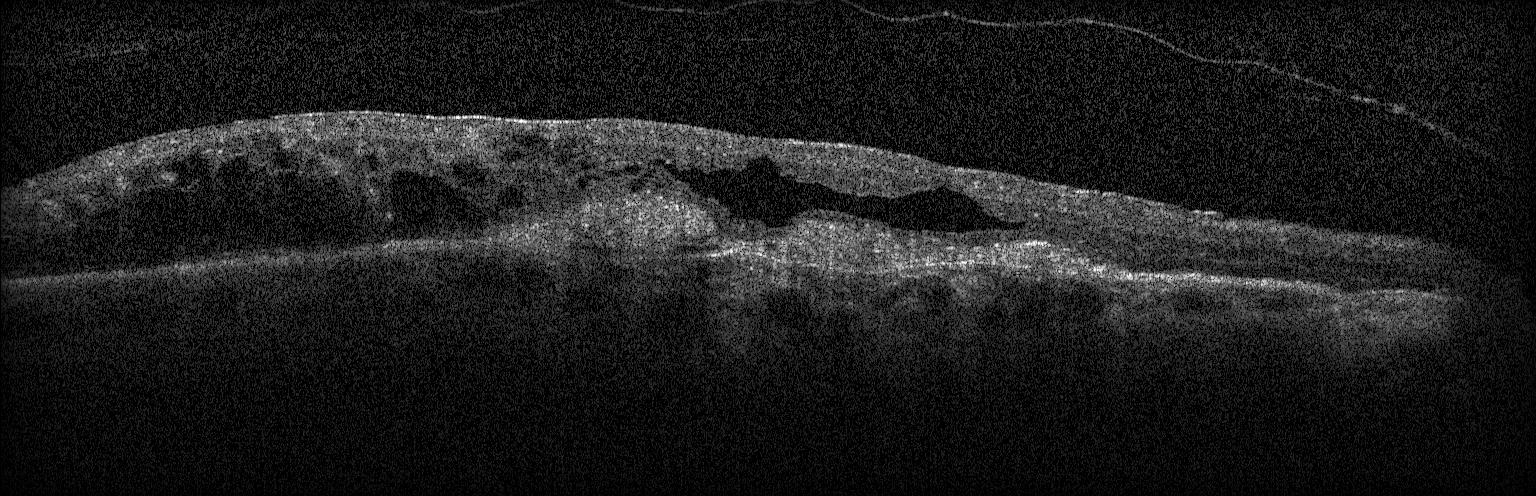 Heidelberg Spectralis OCT system · OCT line scan. Impression: a choroidal neovascular membrane.